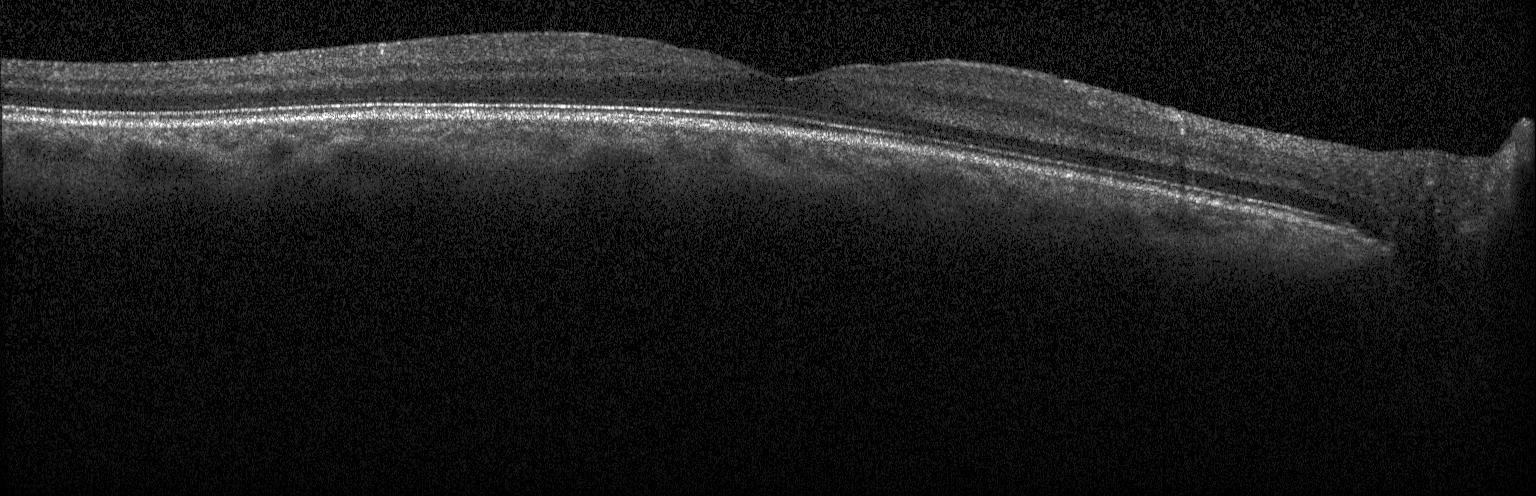
Optical coherence tomography scan. Spectral-domain optical coherence tomography. Impression: no CNV, no DME, and no drusen.